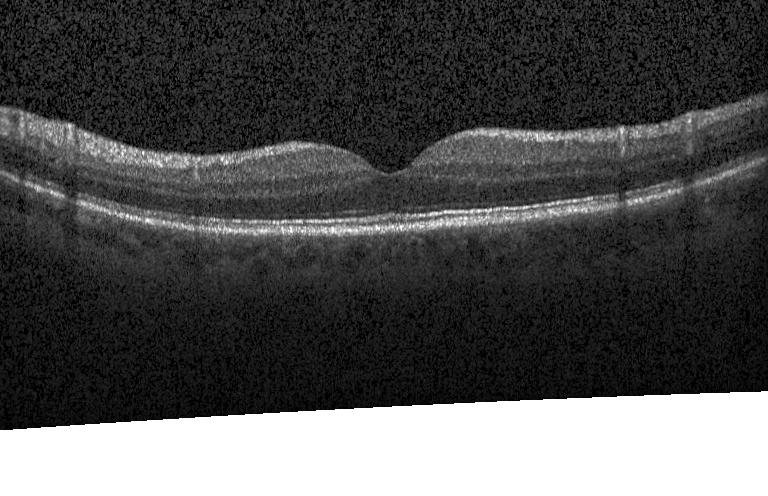 This B-scan demonstrates no choroidal neovascularization, diabetic macular edema, or drusen.